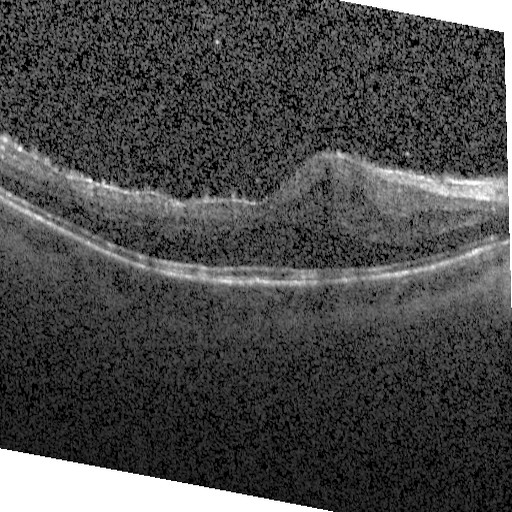
SD-OCT; retinal OCT cross-section; horizontal scan through the fovea; acquired on a Heidelberg Spectralis.
The scan shows DME.